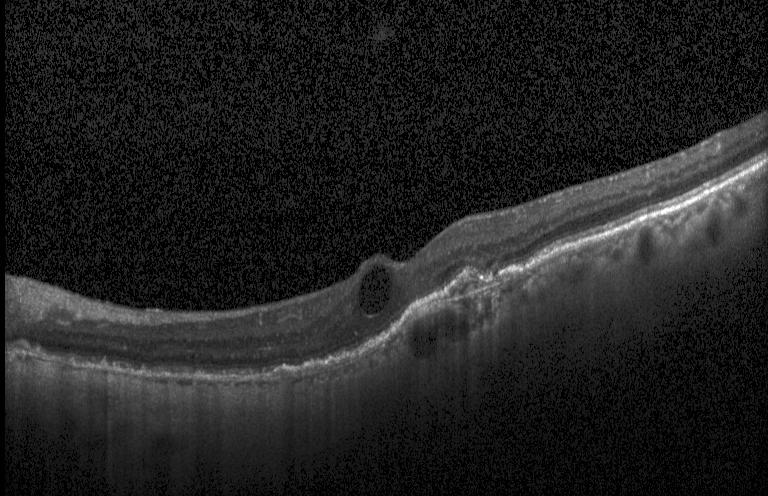

OCT scan showing choroidal neovascularization.